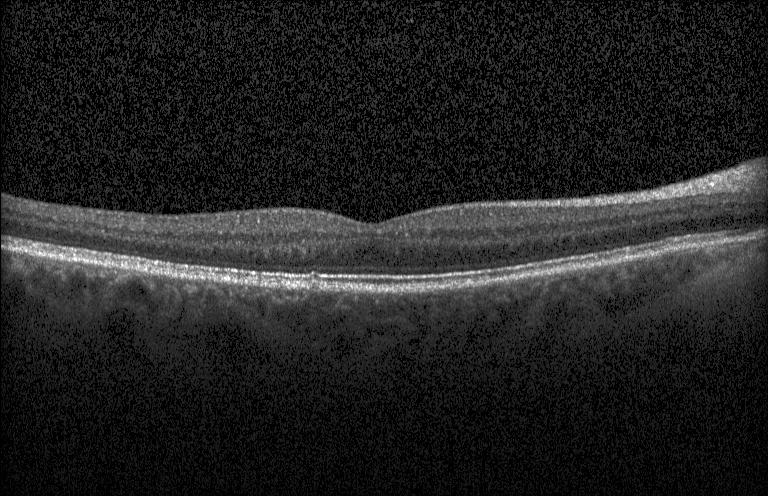 Spectral-domain OCT B-scan: neither choroidal neovascularization, diabetic macular edema, nor drusen.